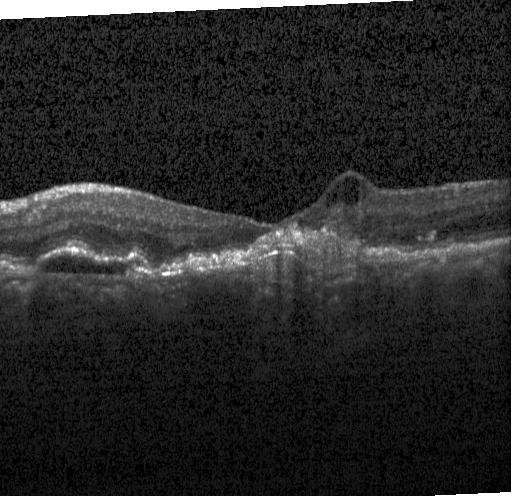
The scan shows choroidal neovascularization.